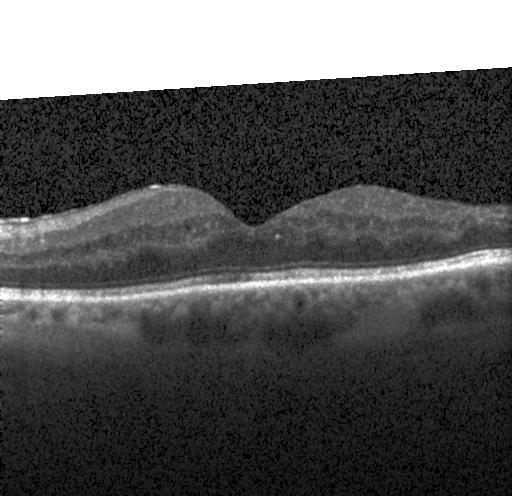

Finding: neither choroidal neovascularization, diabetic macular edema, nor drusen.